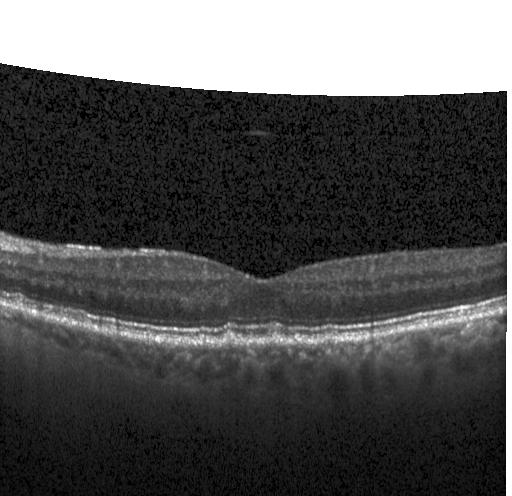 Dx: multiple drusen.